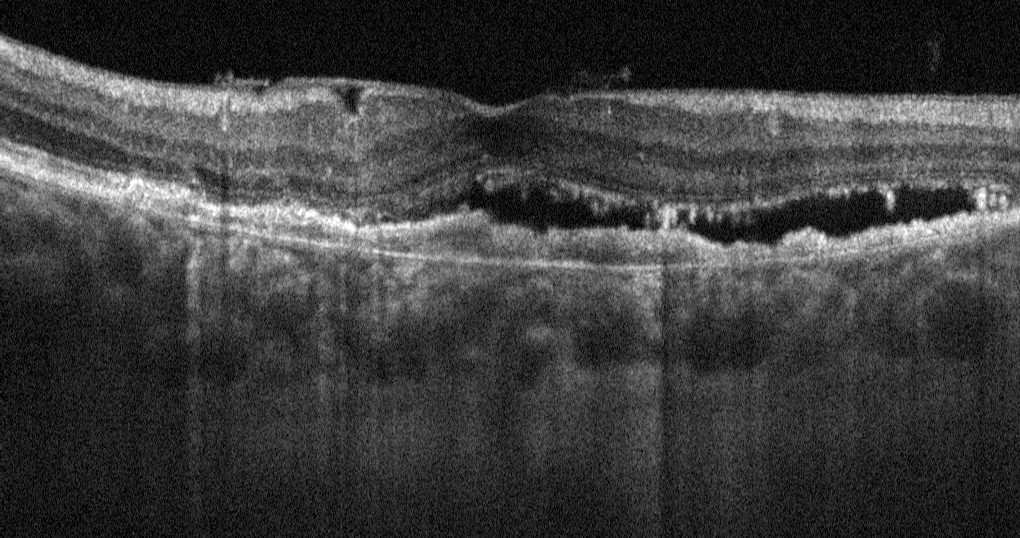
OCT scan showing age-related macular degeneration.